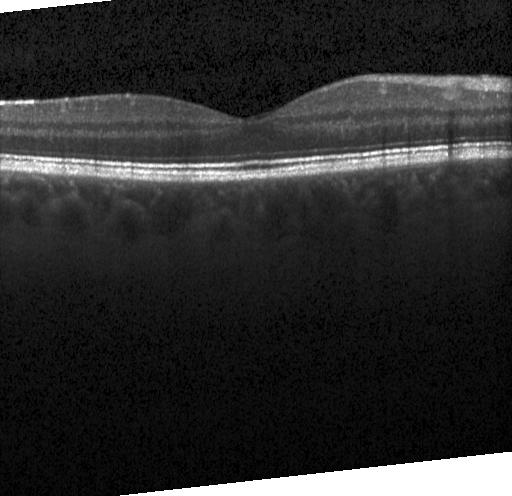 Impression: no choroidal neovascularization, diabetic macular edema, or drusen.